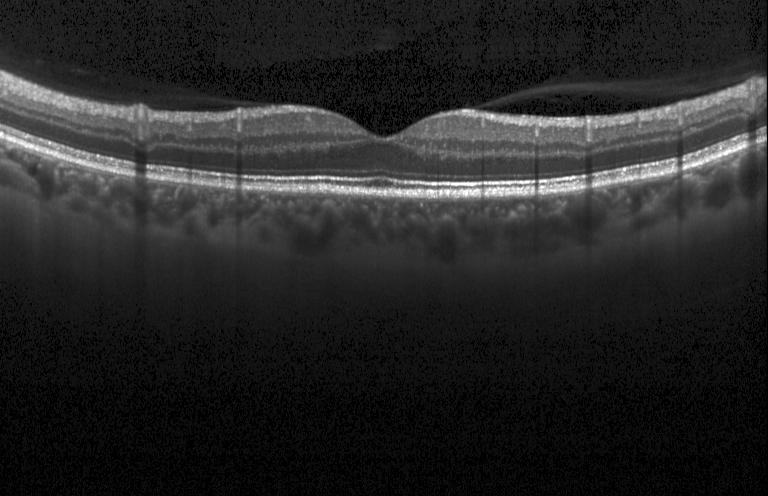

Macular OCT: neither choroidal neovascularization, diabetic macular edema, nor drusen.